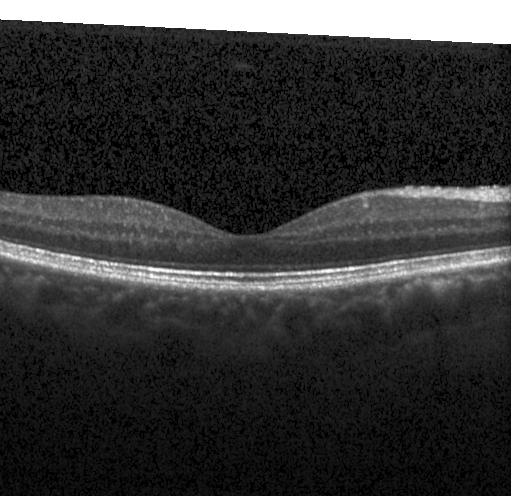
Finding: neither CNV, DME, nor drusen.